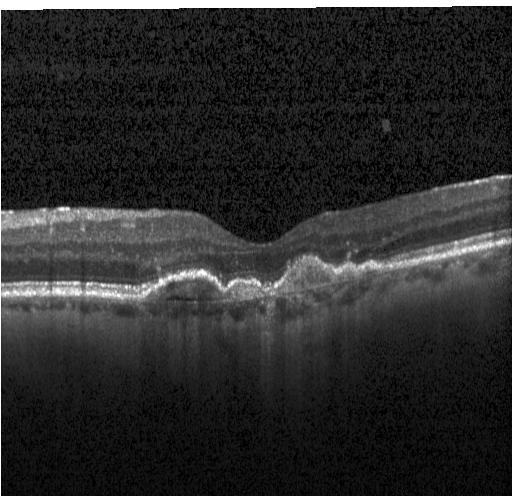 OCT finding: a choroidal neovascular membrane.